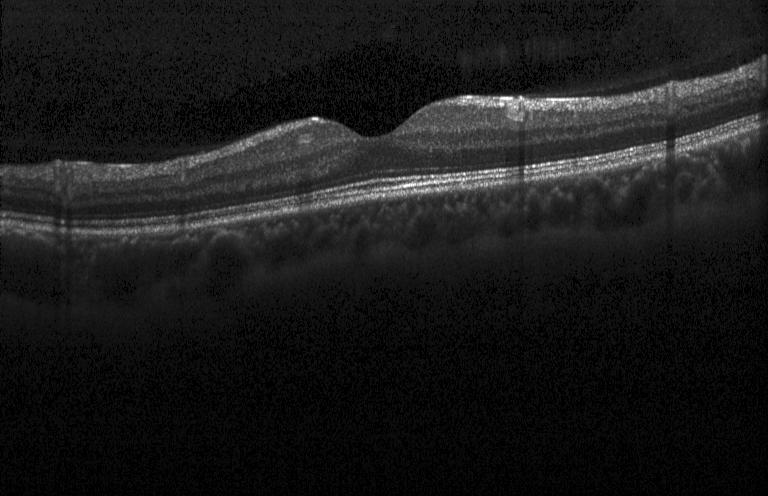 Finding: no choroidal neovascularization, diabetic macular edema, or drusen.